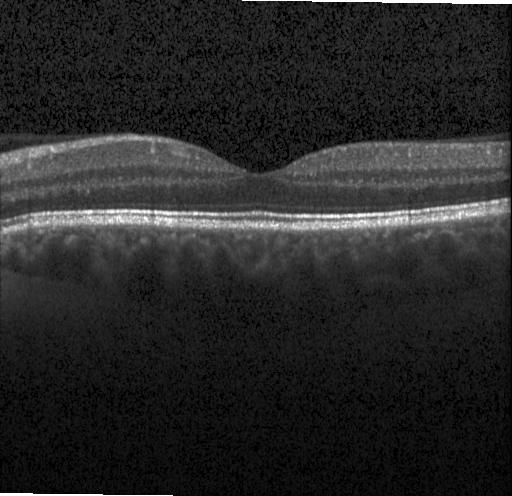 Fovea-centered. Heidelberg Spectralis. Optical coherence tomography B-scan — Diagnosis: no CNV, no DME, and no drusen.